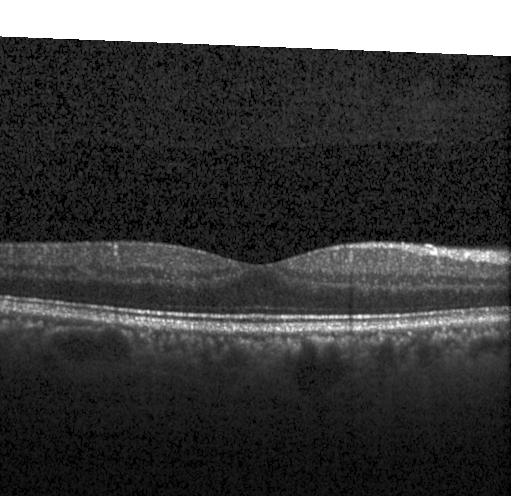 Optical coherence tomography B-scan, fovea-centered, spectral-domain optical coherence tomography
Finding: no evidence of CNV, DME, or drusen.